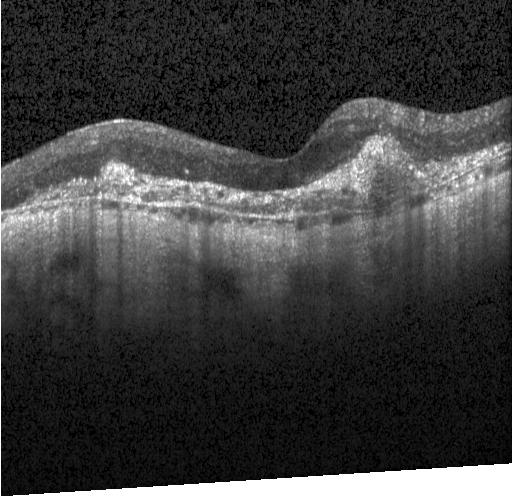

Optical coherence tomography scan — Finding: a choroidal neovascular membrane.